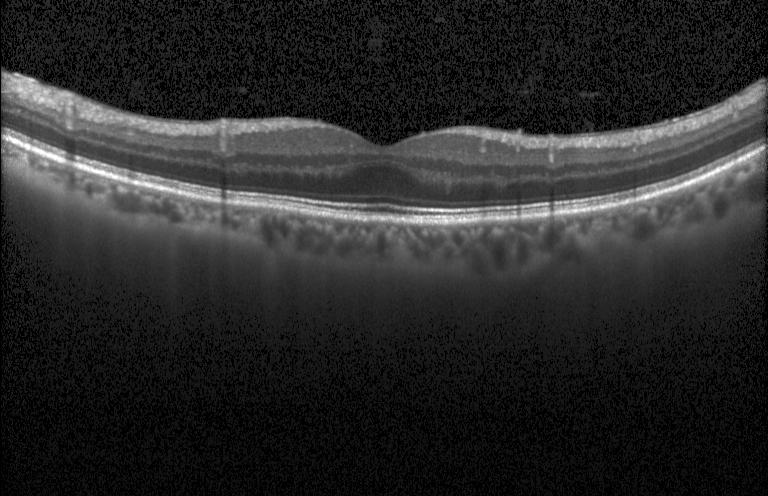

Retinal OCT B-scan; SD-OCT; acquired on a Heidelberg Spectralis
Assessment: no choroidal neovascularization, no diabetic macular edema, and no drusen.